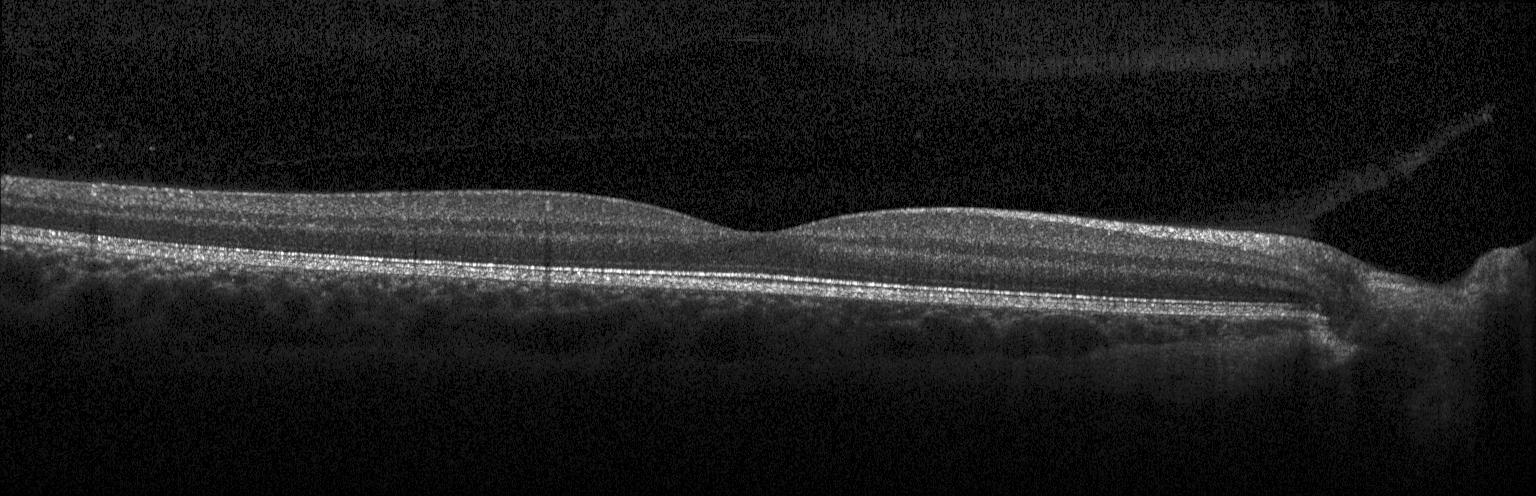
Impression: no evidence of choroidal neovascularization, diabetic macular edema, or drusen.